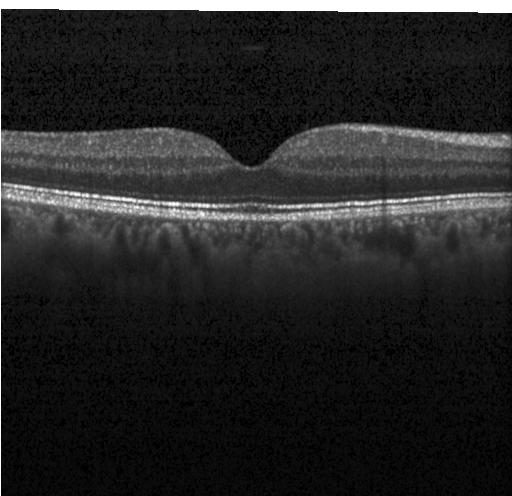
OCT finding: no choroidal neovascularization, diabetic macular edema, or drusen.